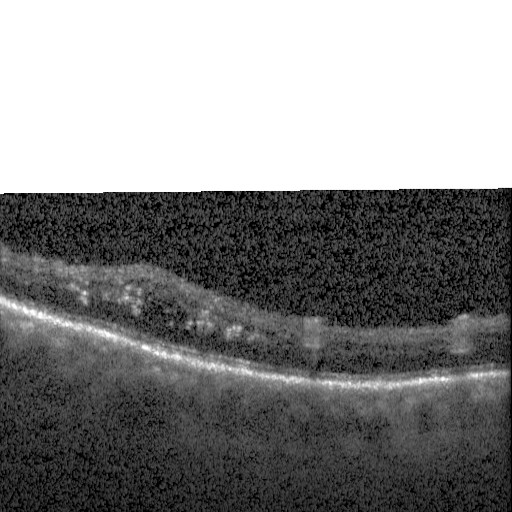

Spectral-domain OCT, Heidelberg Spectralis, horizontal scan through the fovea, retinal OCT B-scan.
Finding: diabetic macular edema.